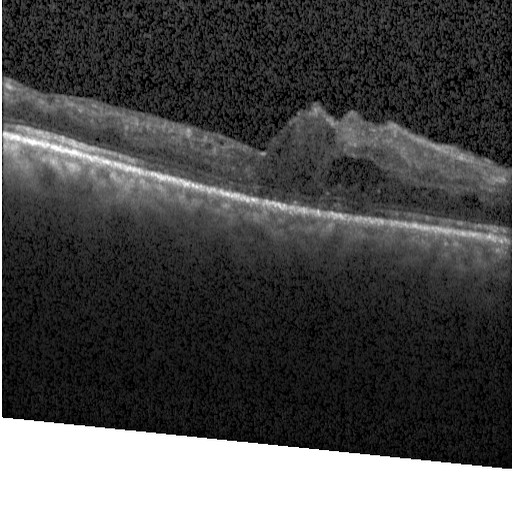 OCT B-scan; spectral-domain OCT; through the macula.
Diagnosis: diabetic macular edema.